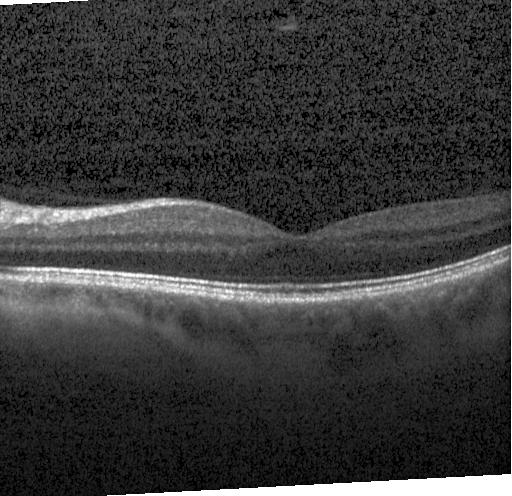 OCT line scan · horizontal scan through the fovea. Impression: no choroidal neovascularization, diabetic macular edema, or drusen.